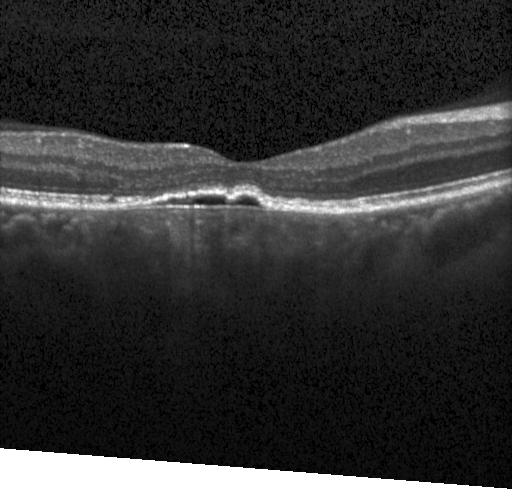
Heidelberg Spectralis OCT system; fovea-centered; OCT B-scan; spectral-domain OCT.
Finding: a choroidal neovascular membrane.